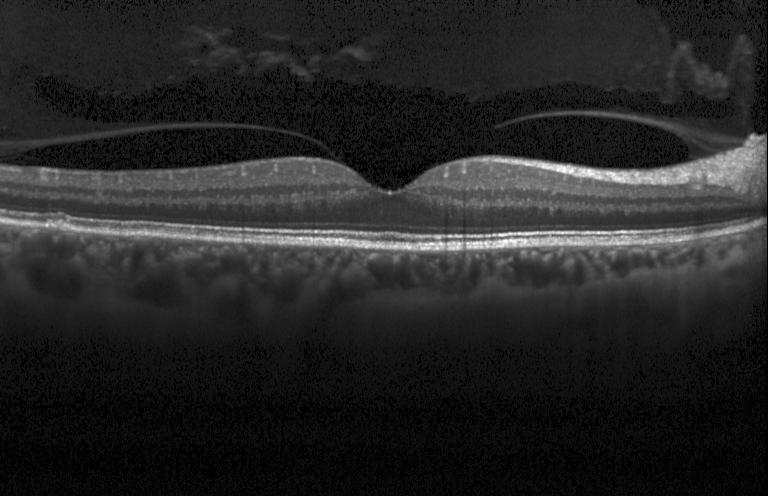 Impression: no evidence of choroidal neovascularization, diabetic macular edema, or drusen.